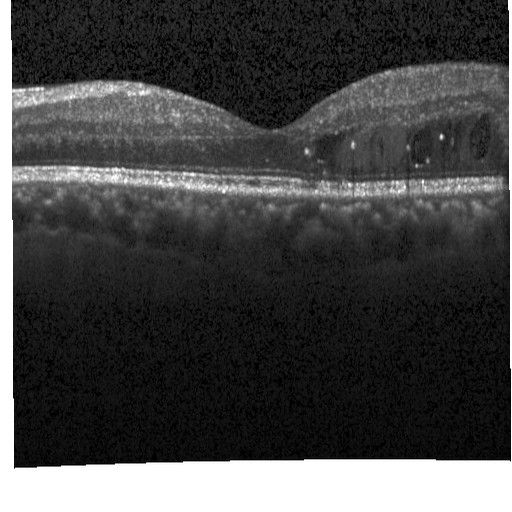
Through the macula. Instrument: Heidelberg Spectralis. Retinal OCT B-scan. Spectral-domain optical coherence tomography. Finding: diabetic macular edema (DME).